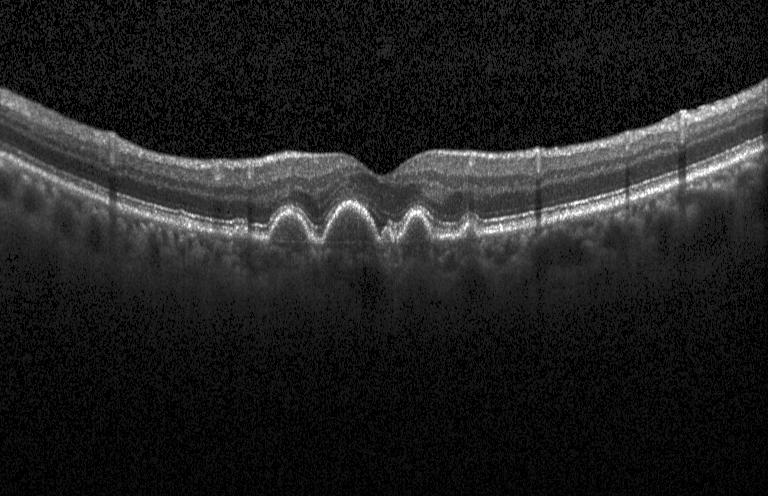

Optical coherence tomography B-scan — Finding: sub-RPE drusenoid deposits.